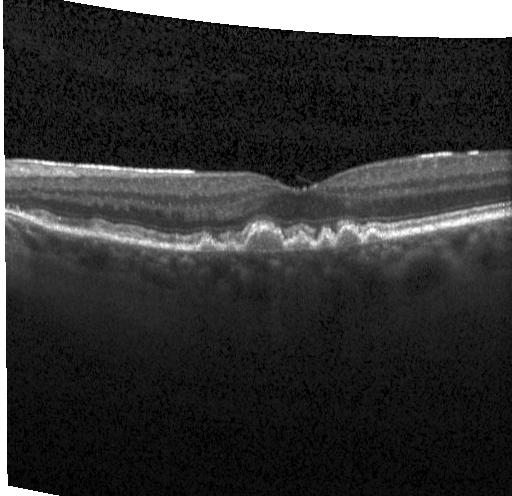
Retinal OCT cross-section
Impression: sub-RPE drusenoid deposits.